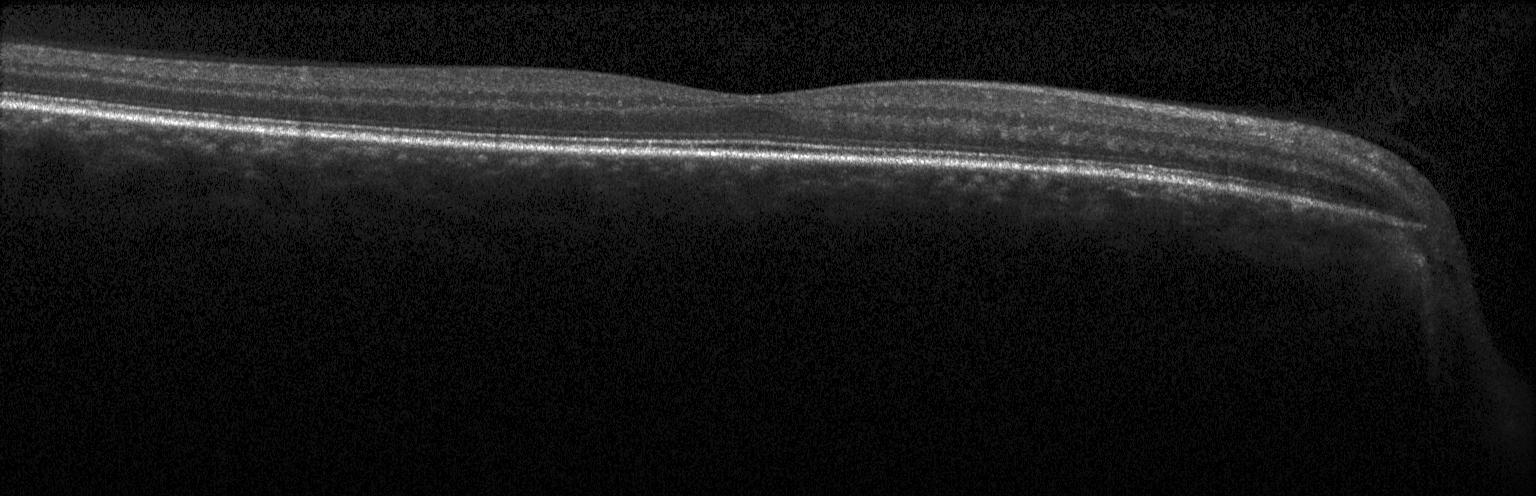
Horizontal scan through the fovea · retinal OCT B-scan. This B-scan demonstrates no evidence of CNV, DME, or drusen.